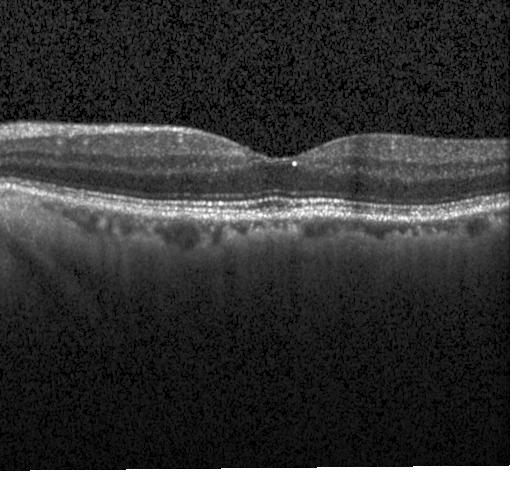 Spectral-domain OCT. Through the macula. Retinal OCT B-scan
Finding: neither choroidal neovascularization, diabetic macular edema, nor drusen.